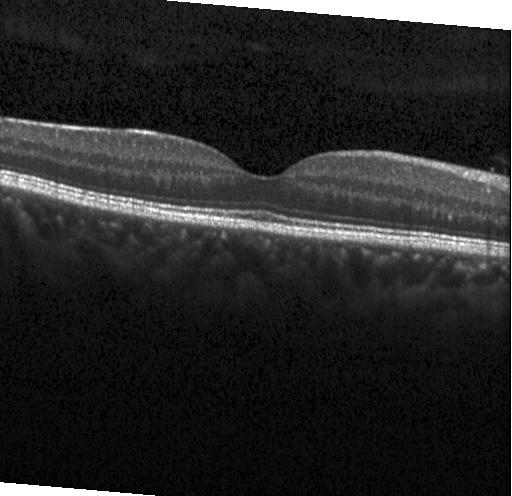
Retinal OCT cross-section · macular scan · spectral-domain optical coherence tomography · acquired on a Heidelberg Spectralis.
Dx: neither choroidal neovascularization, diabetic macular edema, nor drusen.